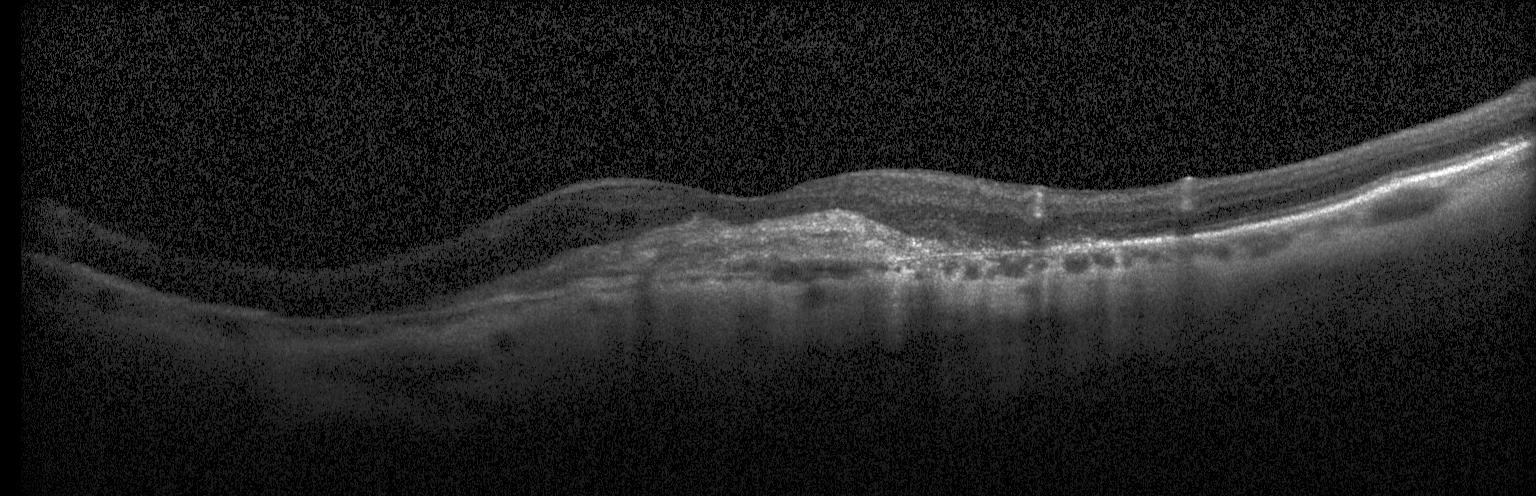
Optical coherence tomography B-scan. Assessment: choroidal neovascularization (CNV).